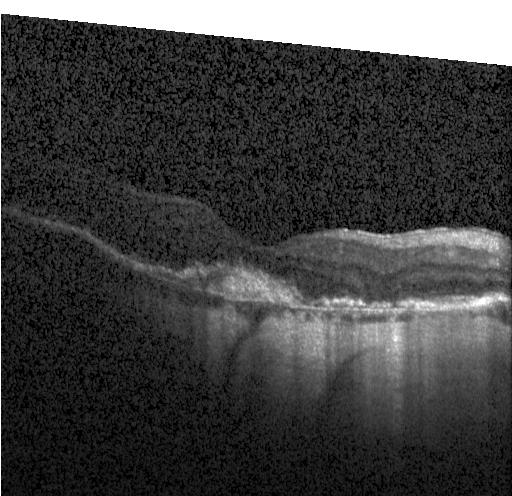
Acquired on a Heidelberg Spectralis. SD-OCT. Retinal OCT B-scan. Centered on the fovea — Choroidal neovascularization.